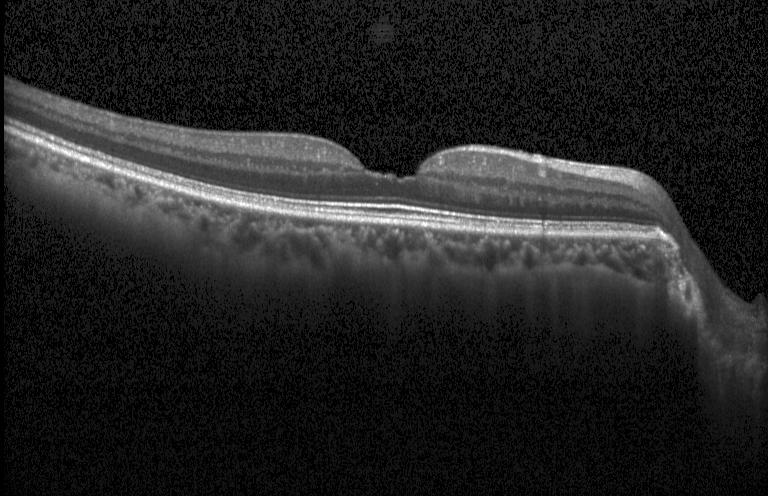

Optical coherence tomography scan
Impression: no evidence of choroidal neovascularization, diabetic macular edema, or drusen.